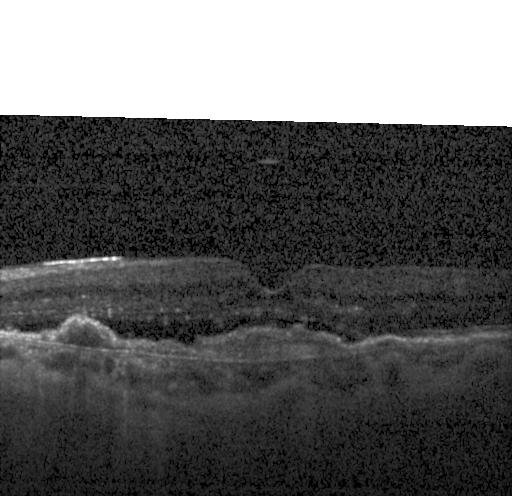

Spectral-domain OCT B-scan: choroidal neovascularization.